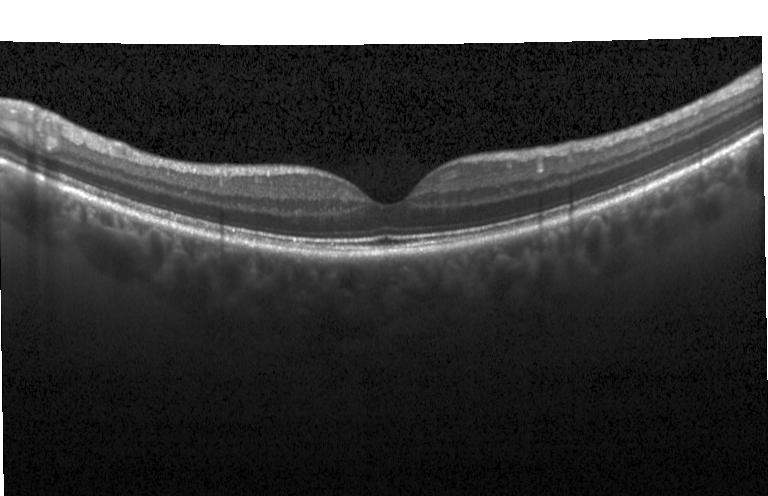

Macular OCT: no choroidal neovascularization, no diabetic macular edema, and no drusen.